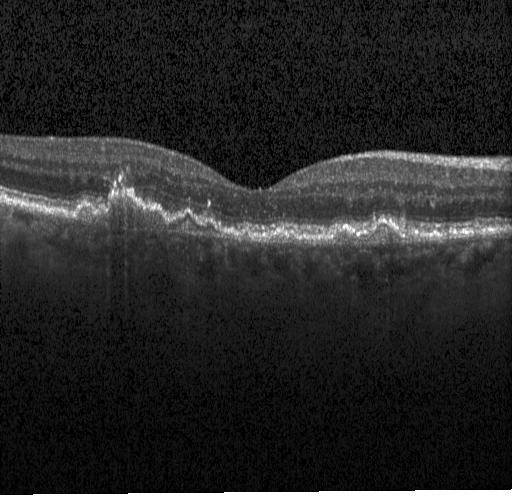
Fovea-centered; retinal OCT B-scan; spectral-domain optical coherence tomography
OCT finding: a choroidal neovascular membrane.